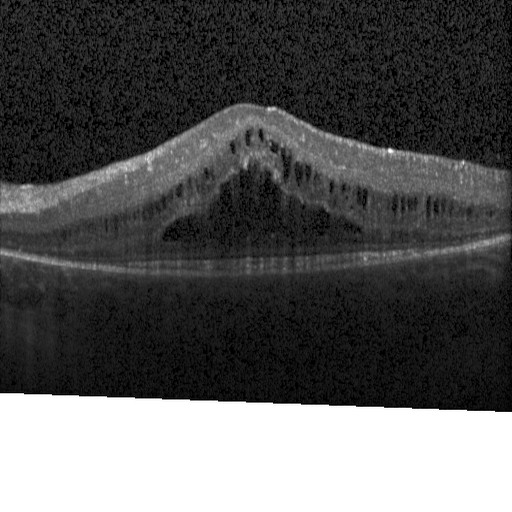 Spectral-domain optical coherence tomography · retinal OCT cross-section
Finding: DME.